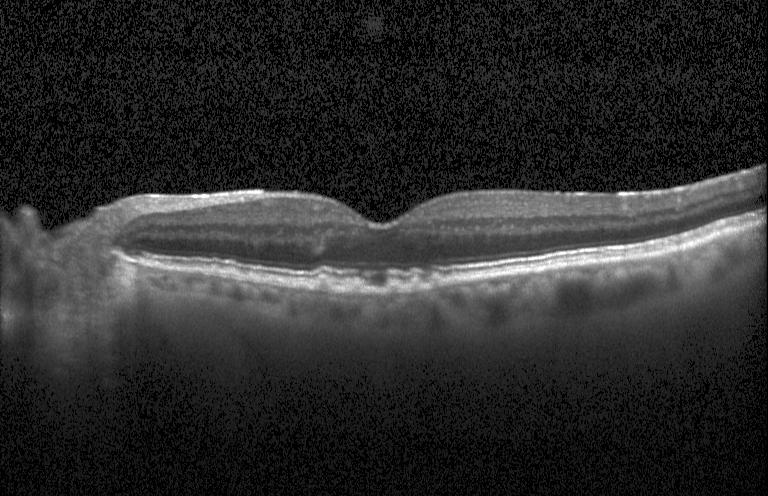
Diagnosis: drusen.